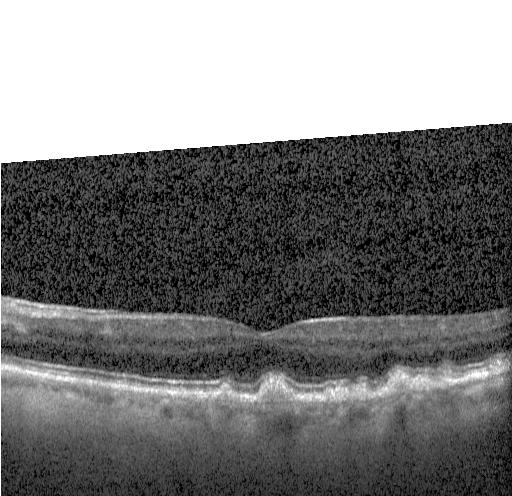
Macular scan, optical coherence tomography B-scan, spectral-domain optical coherence tomography
Finding: sub-RPE drusenoid deposits.